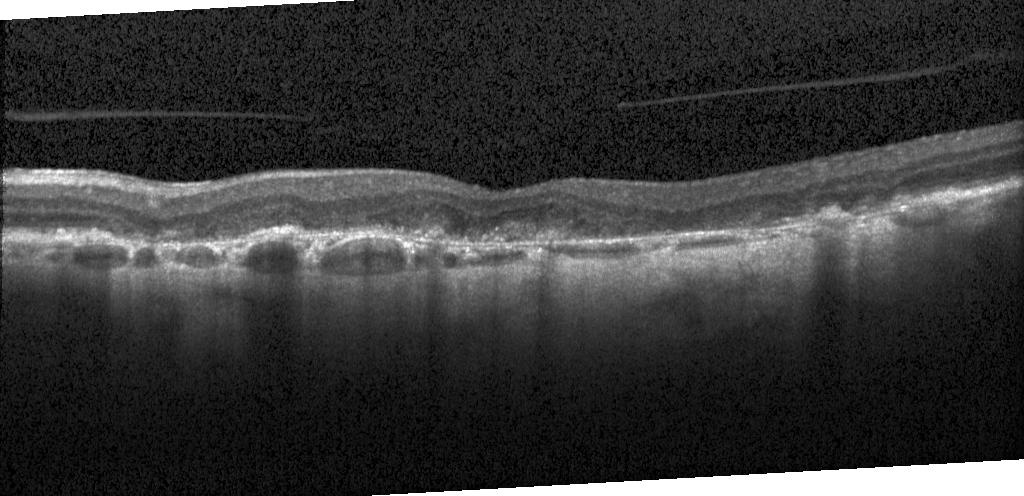 Retinal OCT cross-section, SD-OCT.
Finding: no evidence of choroidal neovascularization, diabetic macular edema, or drusen.